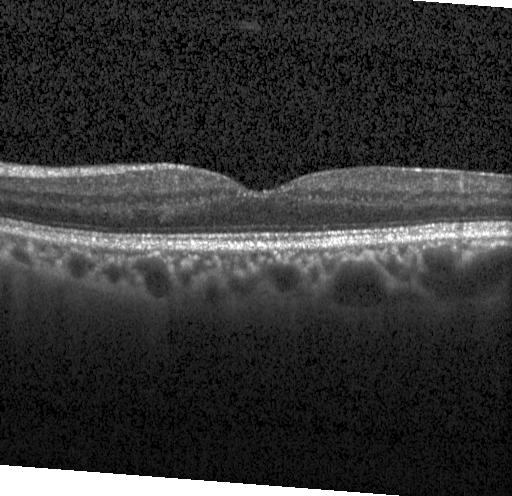

No choroidal neovascularization, diabetic macular edema, or drusen.